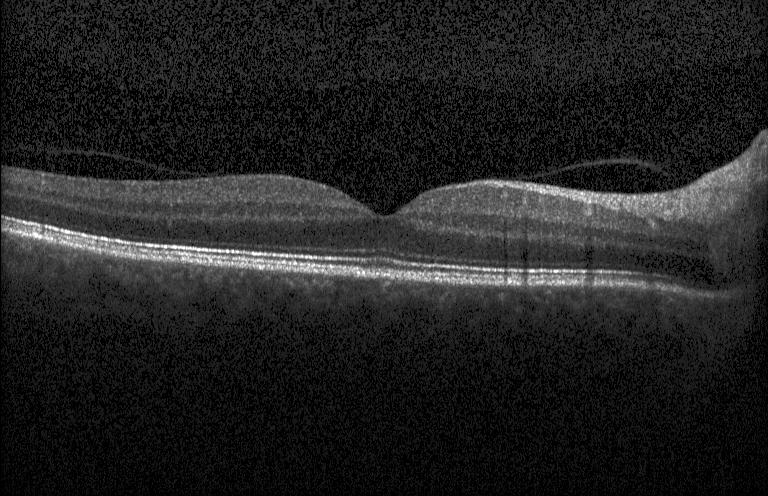 Macular OCT demonstrating neither choroidal neovascularization, diabetic macular edema, nor drusen.